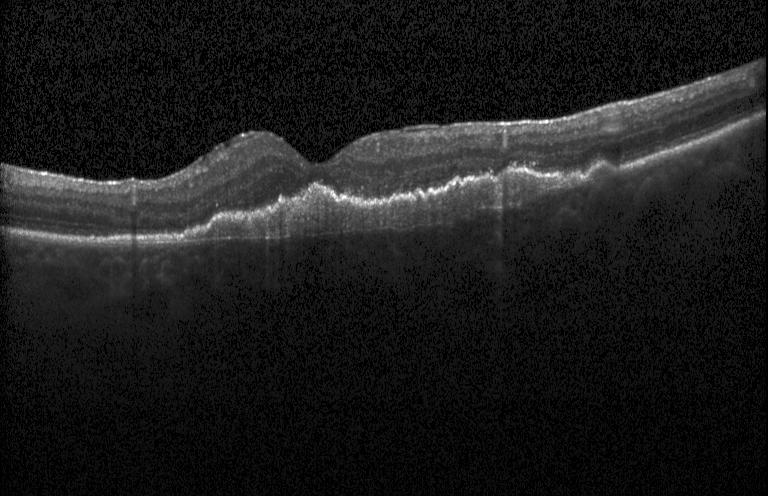
Spectral-domain optical coherence tomography · centered on the fovea · retinal OCT cross-section — Finding: choroidal neovascularization (CNV).